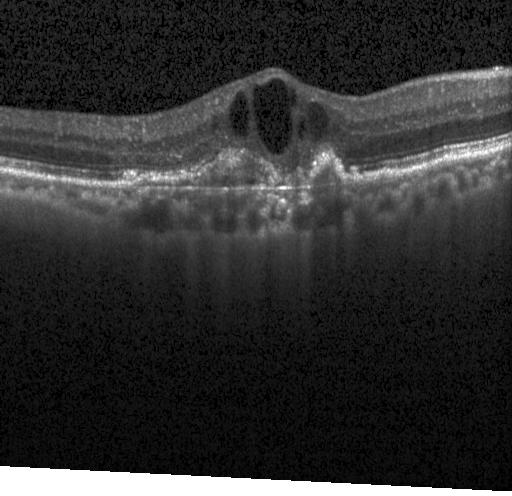
OCT B-scan; spectral-domain optical coherence tomography; centered on the fovea.
Finding: a choroidal neovascular membrane.